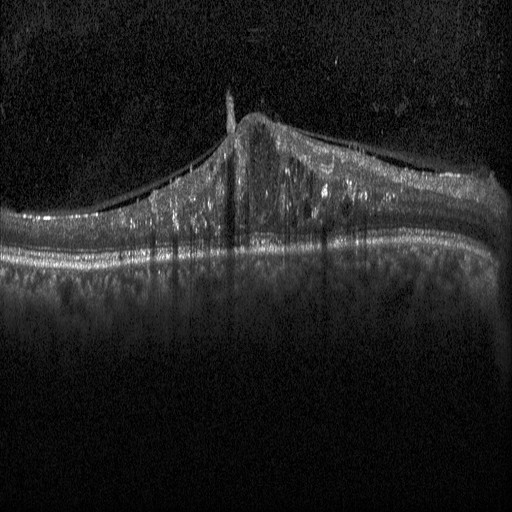

Macular OCT demonstrating diabetic macular edema (DME).